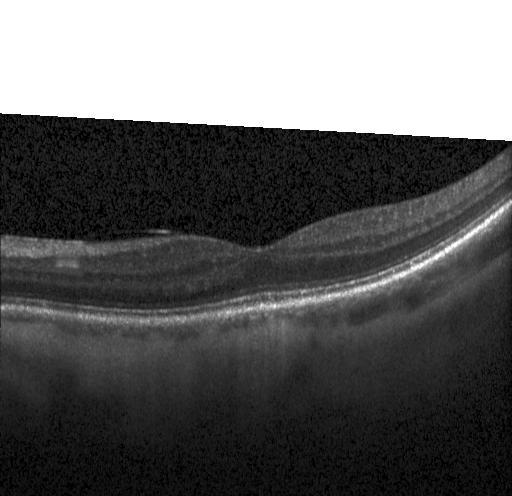
Diagnosis: no evidence of choroidal neovascularization, diabetic macular edema, or drusen.